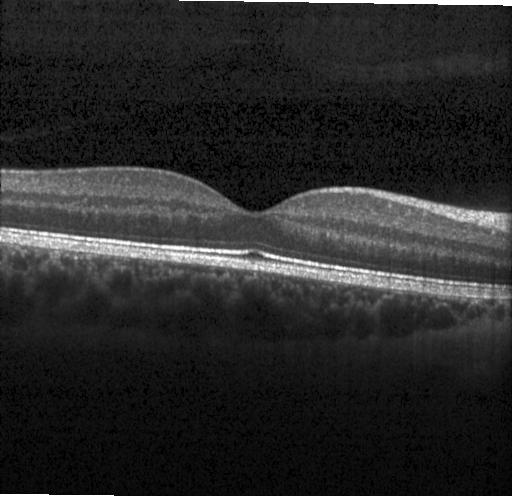 Optical coherence tomography scan. Instrument: Heidelberg Spectralis
The scan shows no choroidal neovascularization, no diabetic macular edema, and no drusen.